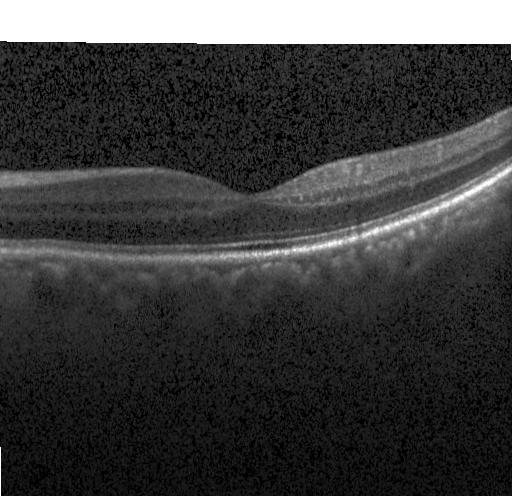

Finding: neither choroidal neovascularization, diabetic macular edema, nor drusen.